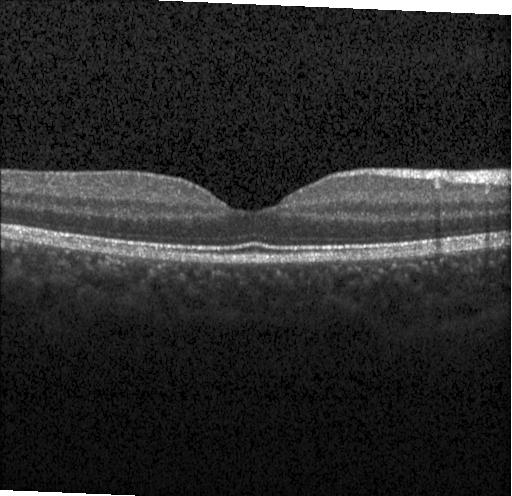 Optical coherence tomography B-scan.
Impression: no choroidal neovascularization, no diabetic macular edema, and no drusen.